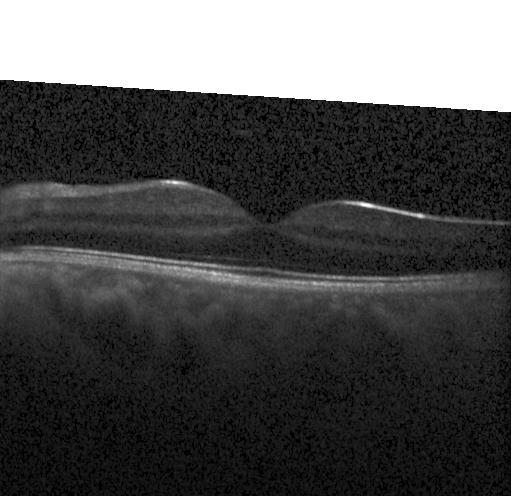
Finding: no evidence of choroidal neovascularization, diabetic macular edema, or drusen.